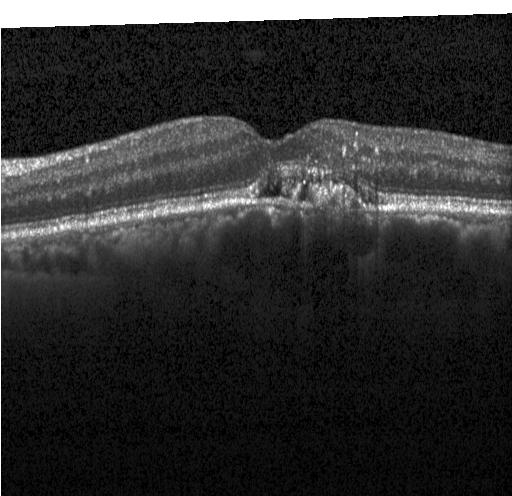
Optical coherence tomography scan — Assessment: choroidal neovascularization.